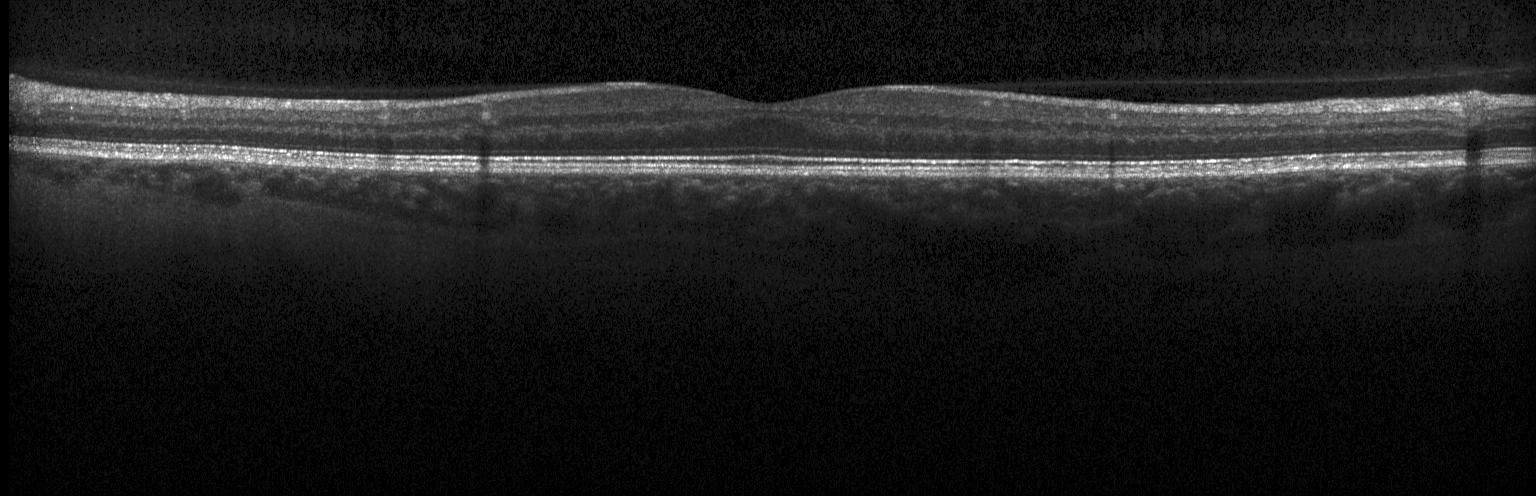
Optical coherence tomography scan; Heidelberg Spectralis OCT system
Macular OCT: neither CNV, DME, nor drusen.